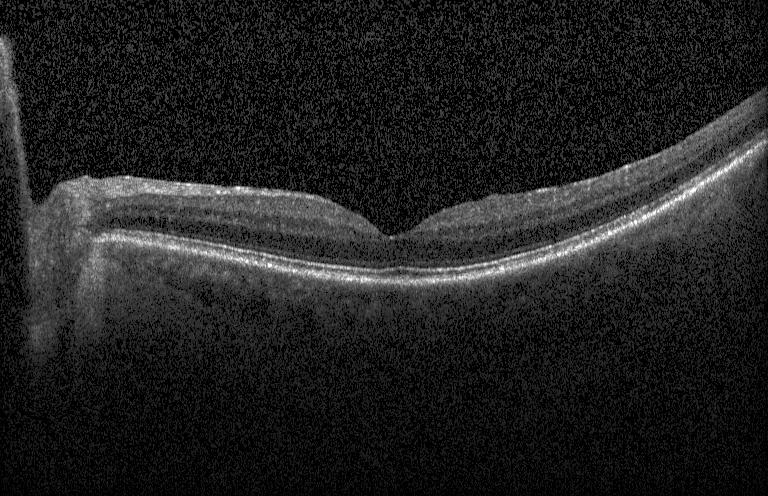
Dx: no evidence of CNV, DME, or drusen.